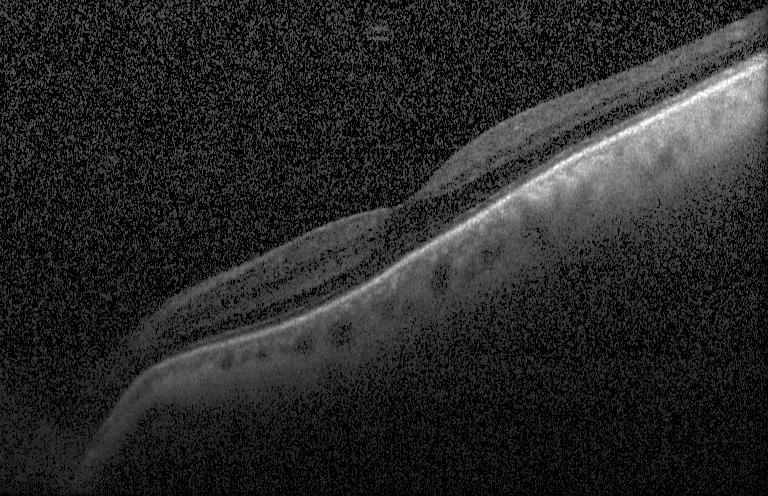

OCT line scan.
The scan shows no choroidal neovascularization, diabetic macular edema, or drusen.